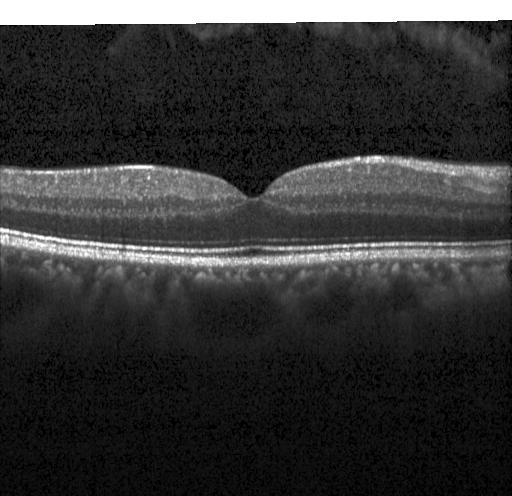

Macular OCT: no evidence of CNV, DME, or drusen.